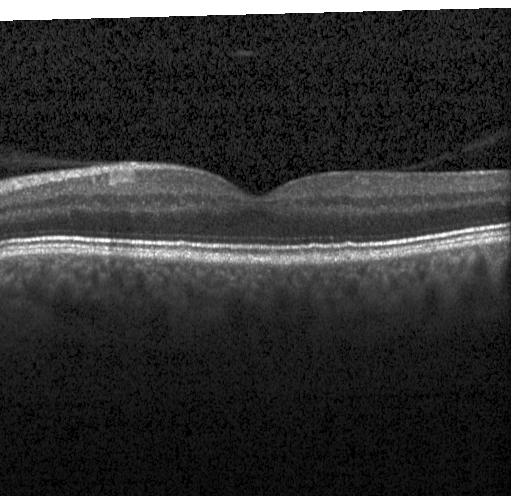
OCT scan showing no choroidal neovascularization, diabetic macular edema, or drusen.